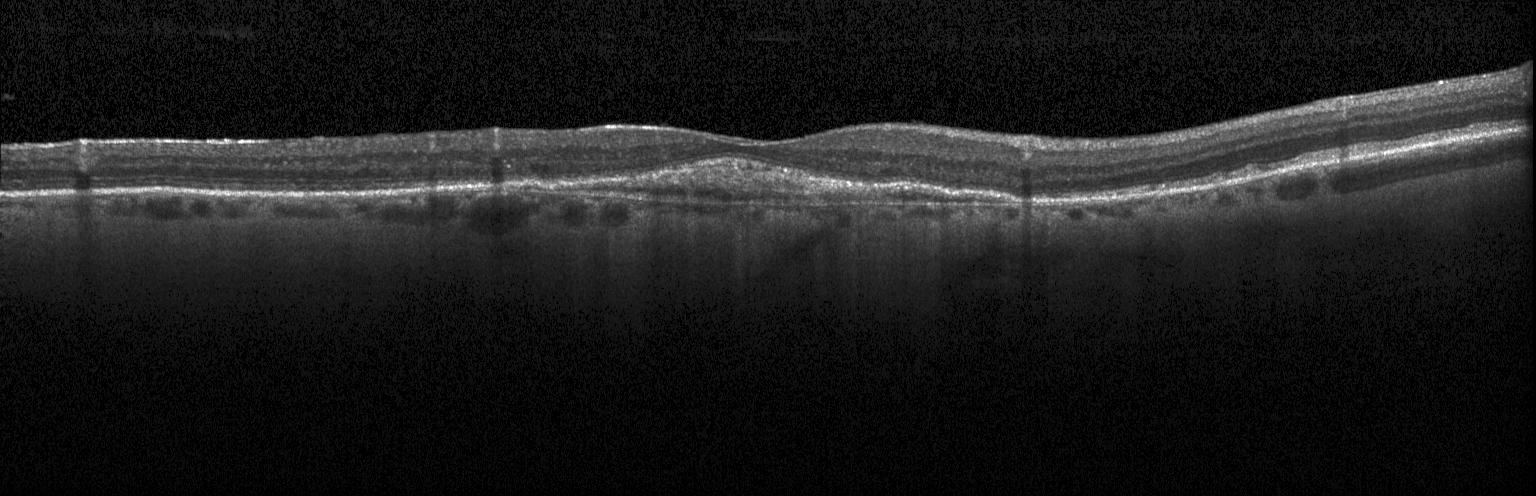
Fovea-centered. OCT B-scan. SD-OCT — This B-scan demonstrates a choroidal neovascular membrane.